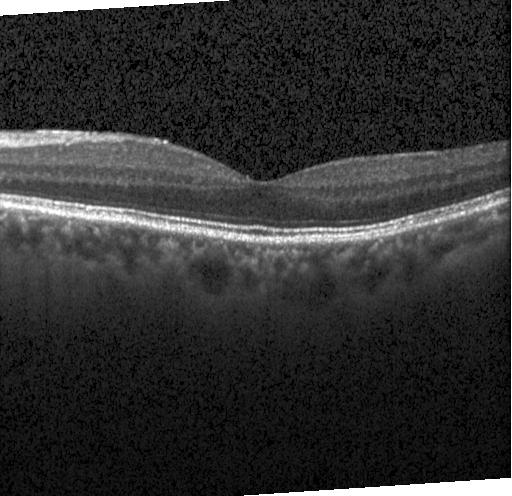
Spectral-domain optical coherence tomography; centered on the fovea; OCT B-scan; Heidelberg Spectralis OCT system. Finding: no choroidal neovascularization, diabetic macular edema, or drusen.